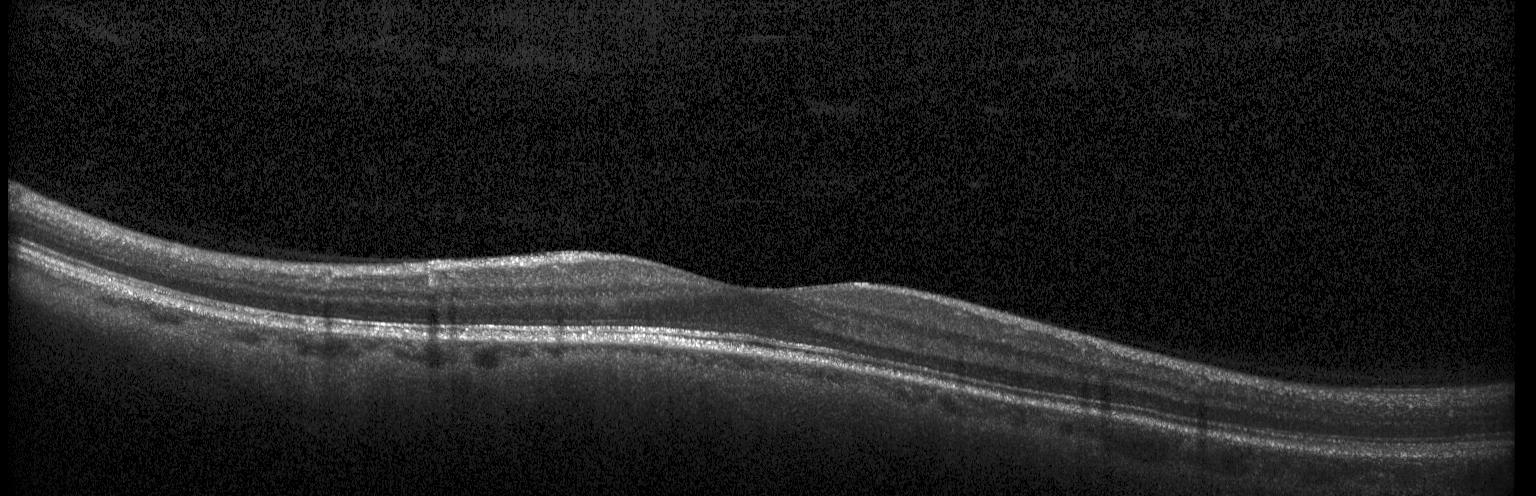

Heidelberg Spectralis · through the macula · spectral-domain OCT · OCT B-scan
Dx: no choroidal neovascularization, no diabetic macular edema, and no drusen.